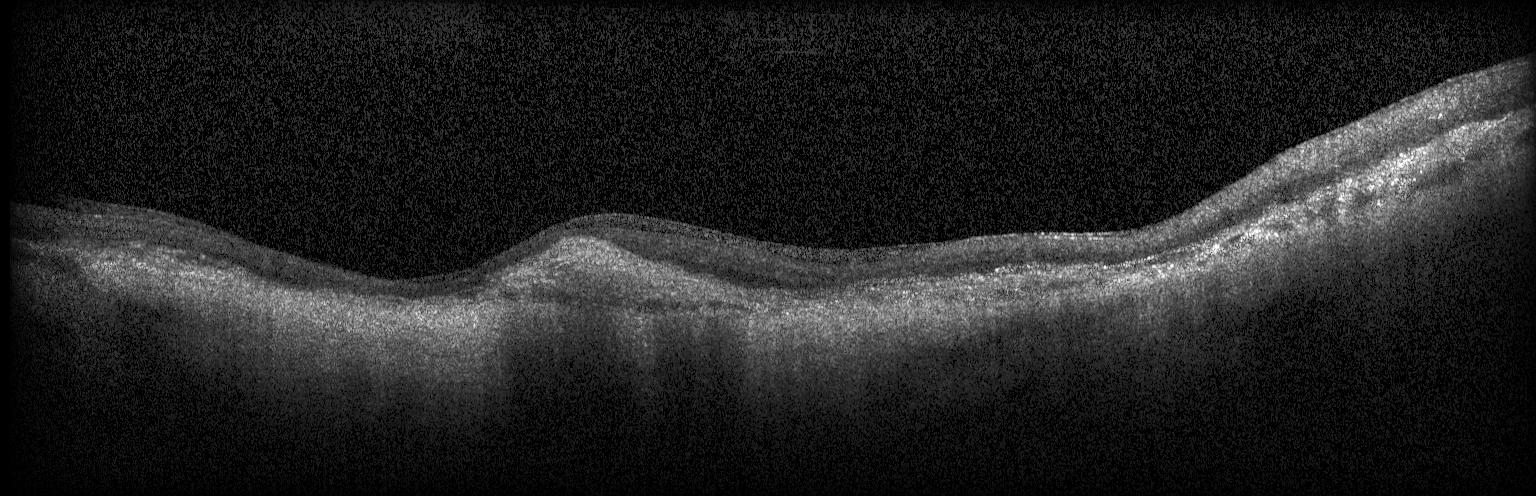
OCT finding: a choroidal neovascular membrane.